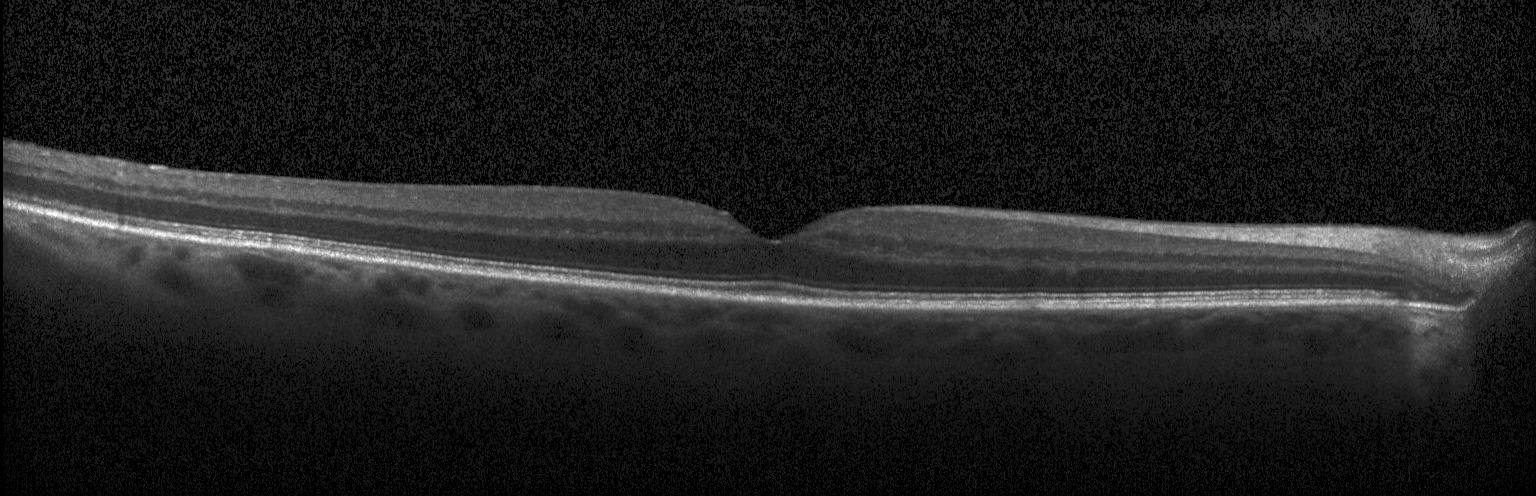 SD-OCT; OCT B-scan; centered on the fovea — Impression: no CNV, DME, or drusen.